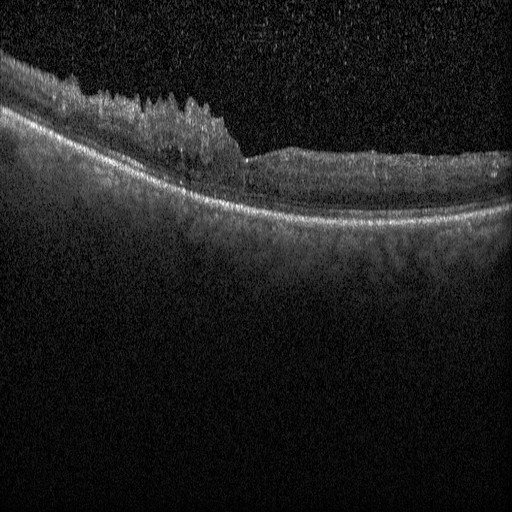 Macular scan · spectral-domain OCT · optical coherence tomography B-scan · Heidelberg Spectralis OCT system. Impression: DME.